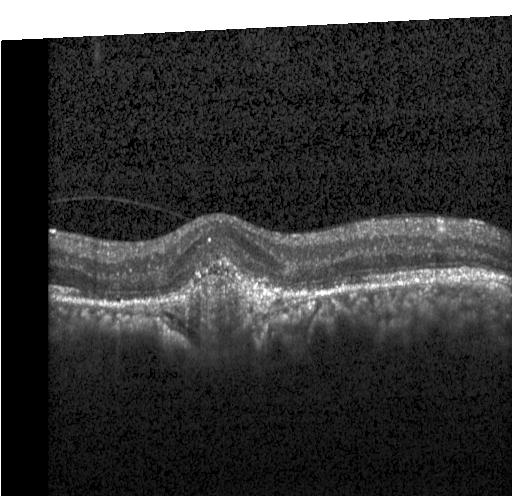
Diagnosis: CNV.